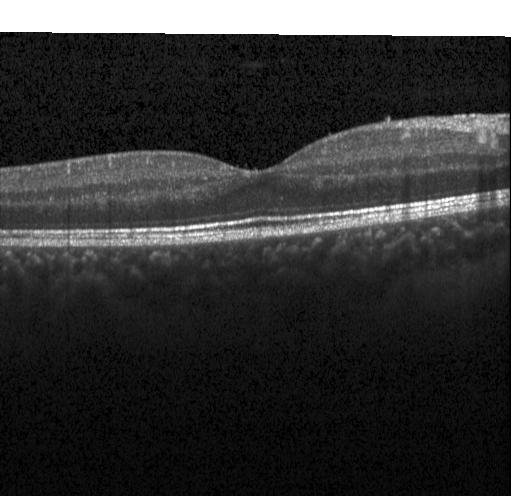 Retinal OCT cross-section
Dx: no choroidal neovascularization, diabetic macular edema, or drusen.